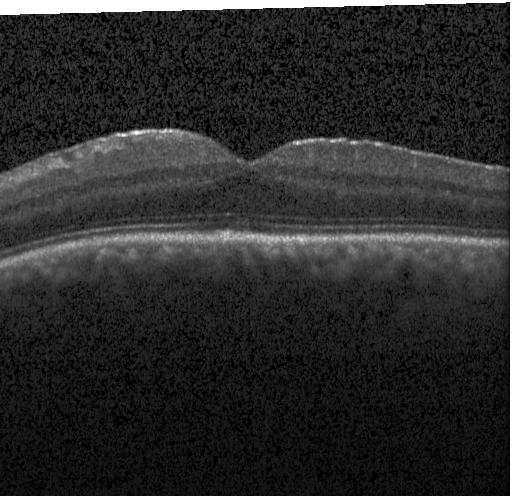

Retinal OCT cross-section. Finding: neither choroidal neovascularization, diabetic macular edema, nor drusen.